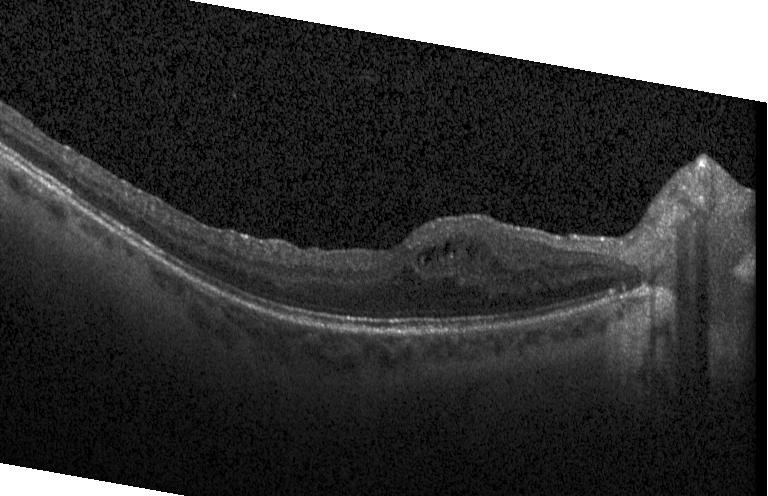

Diagnosis: diabetic macular edema (DME).